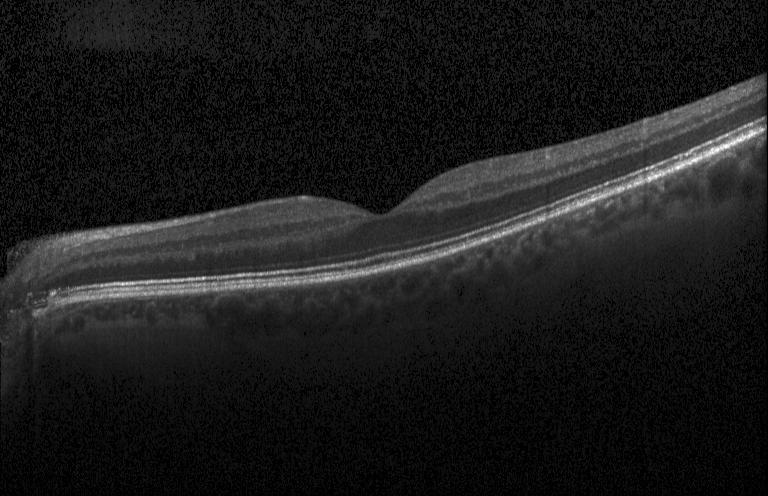

OCT line scan. Diagnosis: neither choroidal neovascularization, diabetic macular edema, nor drusen.